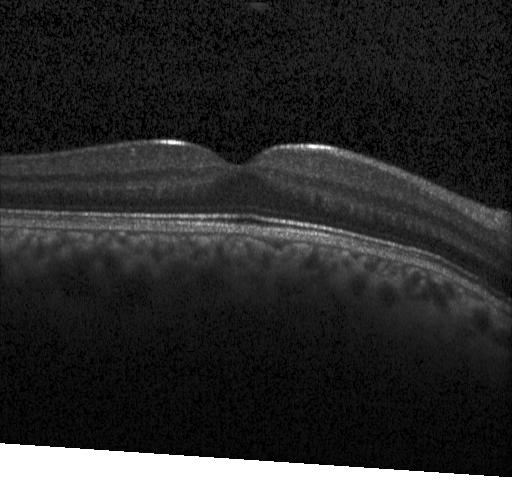

Through the macula; Heidelberg Spectralis OCT system; optical coherence tomography B-scan; spectral-domain optical coherence tomography.
Assessment: neither choroidal neovascularization, diabetic macular edema, nor drusen.